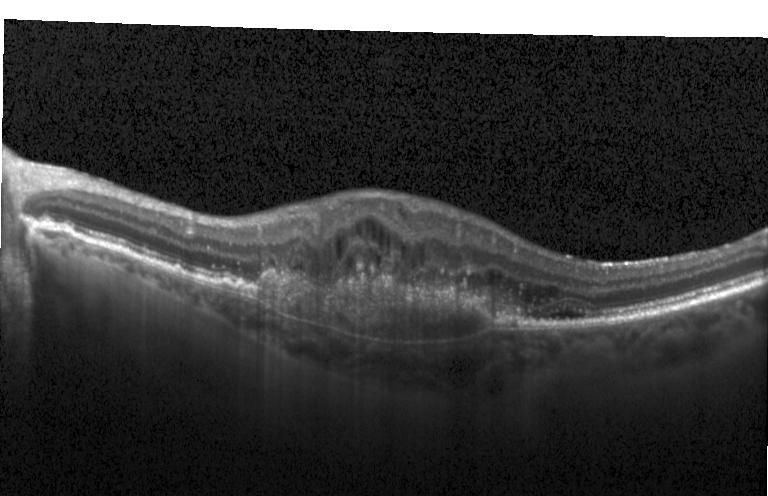 Instrument: Heidelberg Spectralis. SD-OCT. OCT line scan. Through the macula. Finding: choroidal neovascularization (CNV).